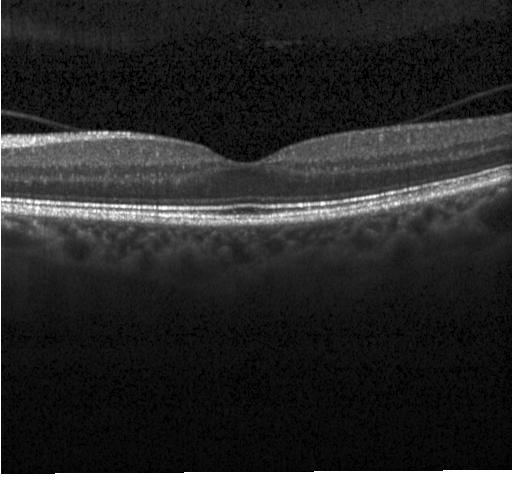
Retinal OCT cross-section showing neither choroidal neovascularization, diabetic macular edema, nor drusen.